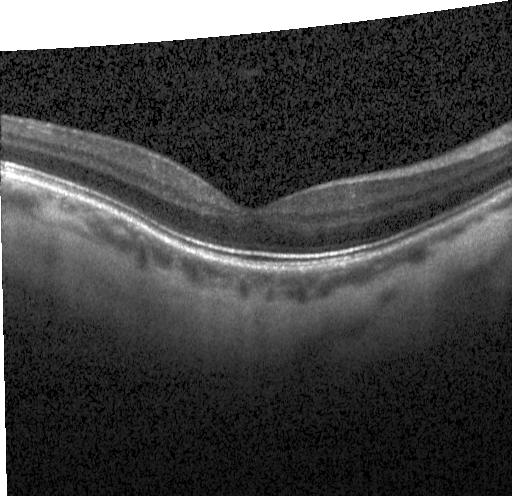

Centered on the fovea, retinal OCT B-scan, SD-OCT.
Impression: no evidence of choroidal neovascularization, diabetic macular edema, or drusen.